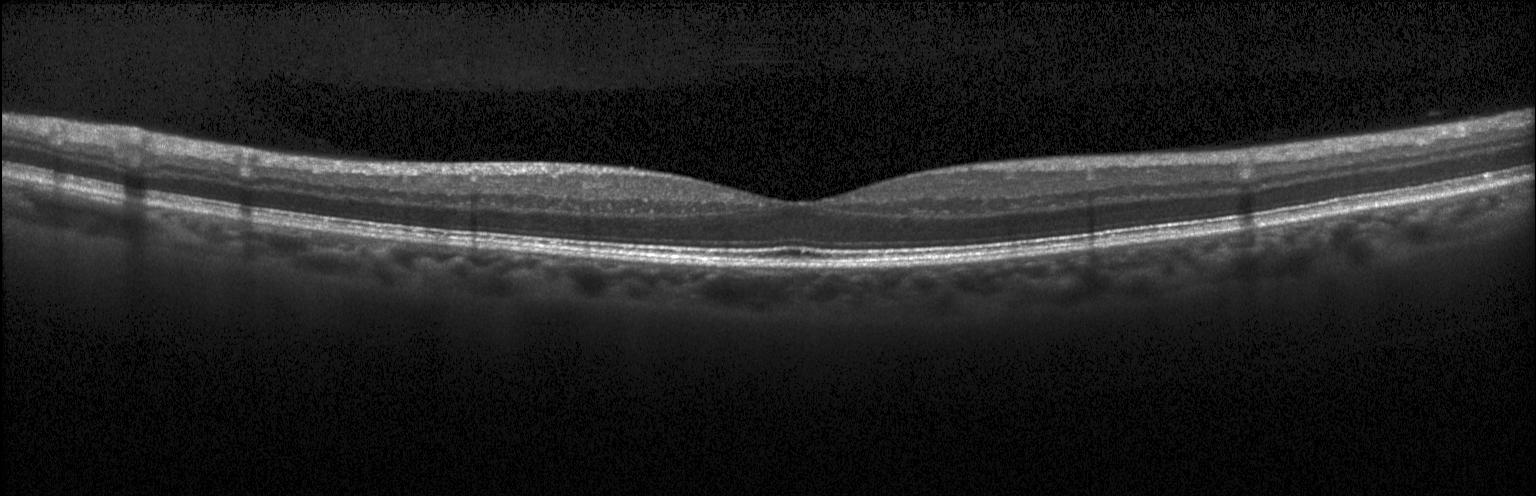
Spectral-domain optical coherence tomography. Optical coherence tomography B-scan — Impression: no choroidal neovascularization, diabetic macular edema, or drusen.